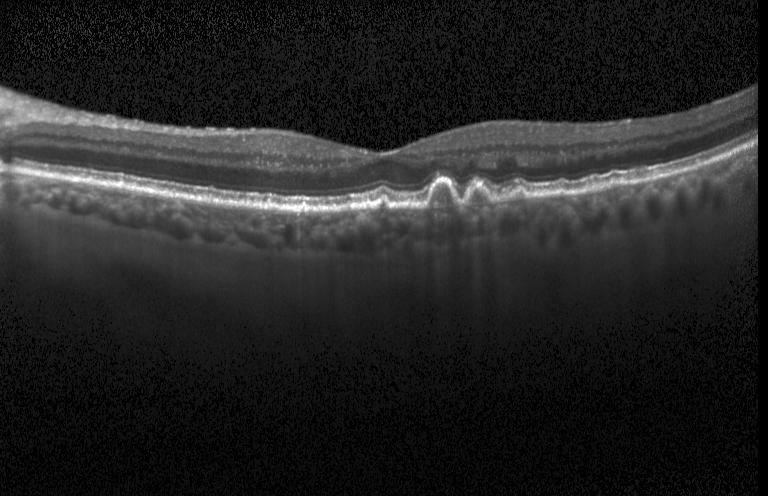
OCT scan showing sub-RPE drusenoid deposits.